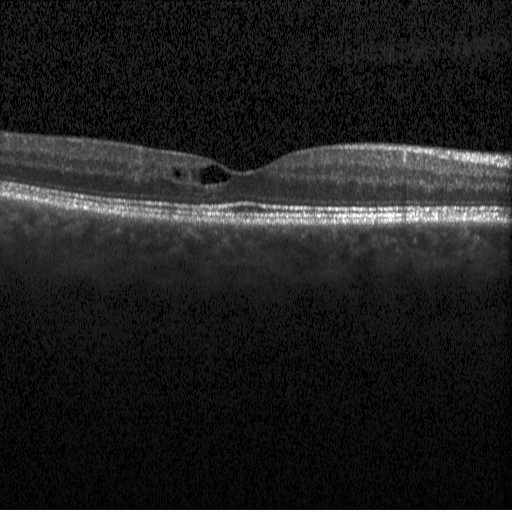 Retinal OCT B-scan · instrument: Heidelberg Spectralis · fovea-centered · SD-OCT — Diagnosis: diabetic macular edema (DME).